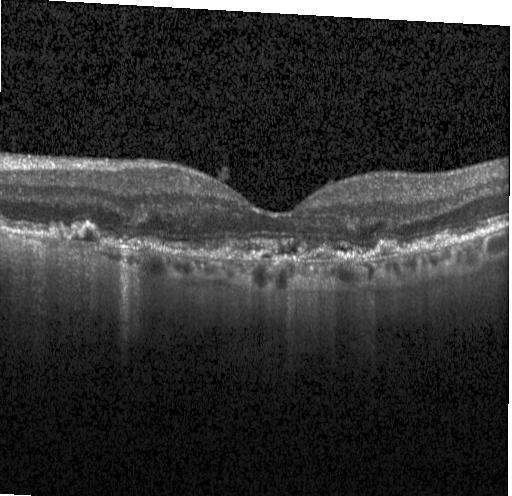
Retinal OCT cross-section — Dx: choroidal neovascularization.